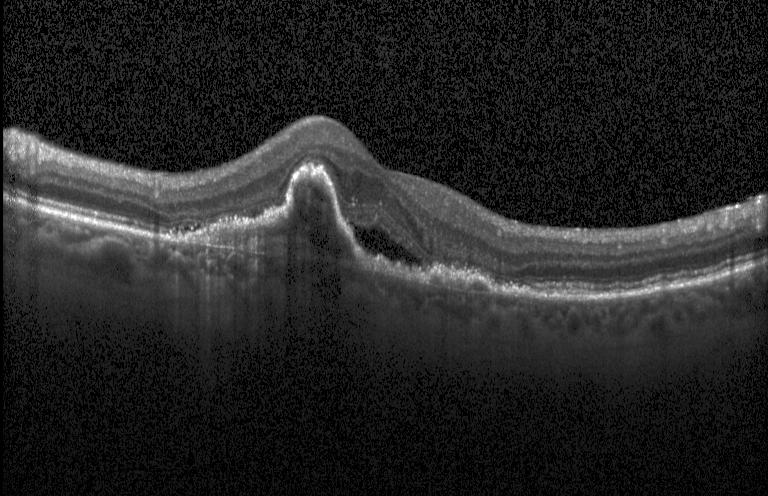
Heidelberg Spectralis · through the macula · optical coherence tomography B-scan · spectral-domain optical coherence tomography.
This B-scan demonstrates a choroidal neovascular membrane.